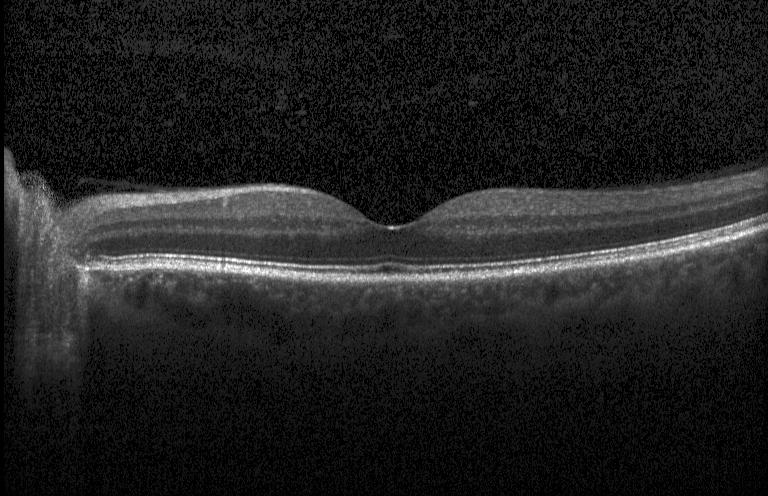
Finding: no choroidal neovascularization, diabetic macular edema, or drusen.